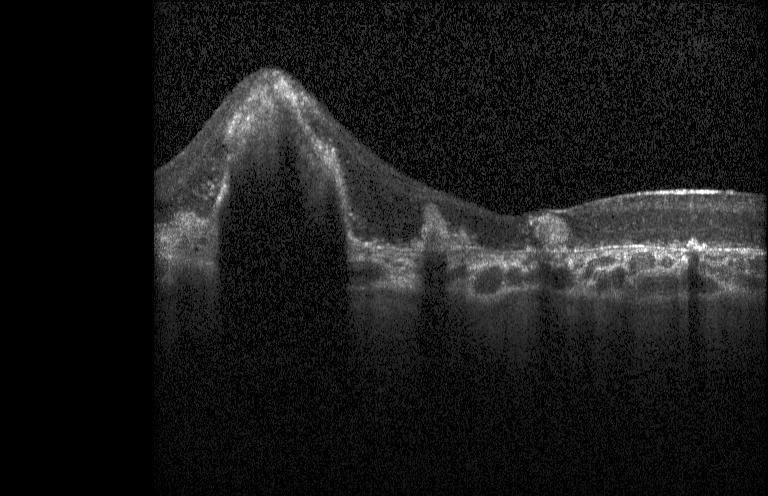

Optical coherence tomography B-scan
This B-scan demonstrates a choroidal neovascular membrane.